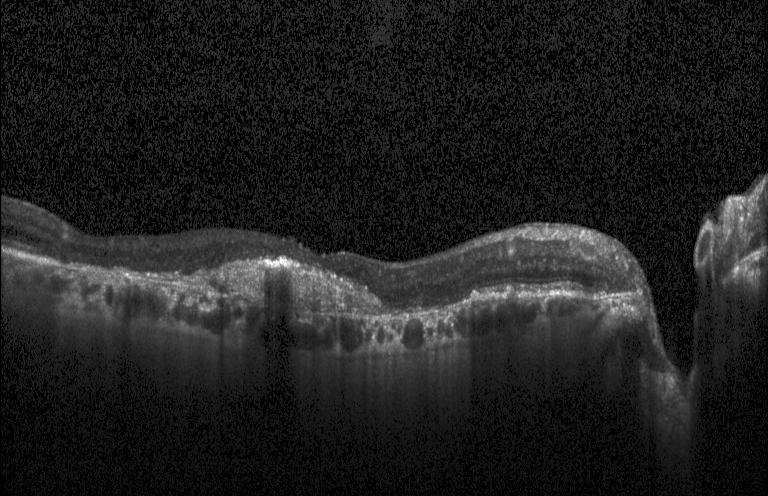
Retinal OCT cross-section showing choroidal neovascularization.